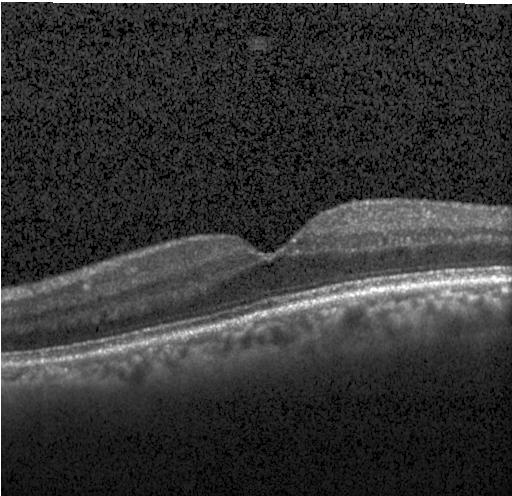
This B-scan demonstrates no CNV, no DME, and no drusen.